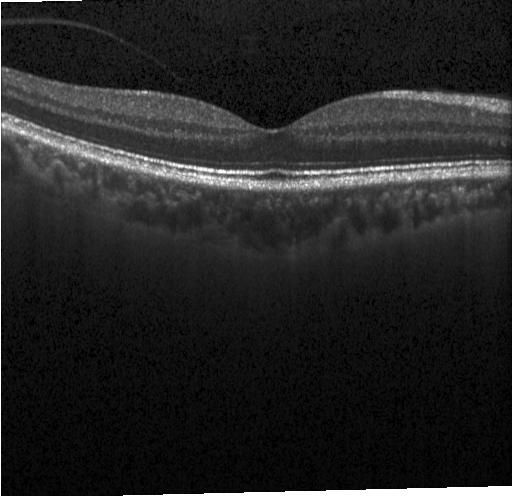

OCT finding: no evidence of choroidal neovascularization, diabetic macular edema, or drusen.